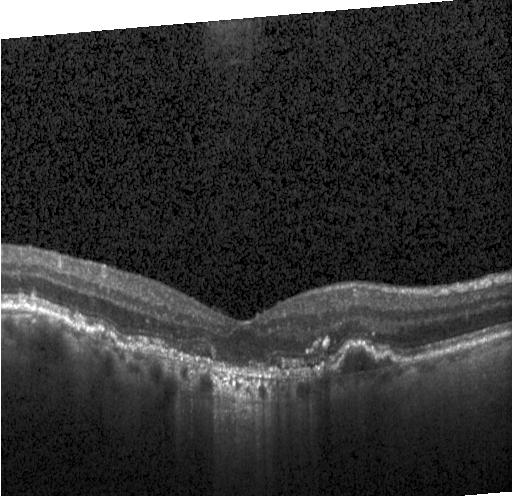 OCT scan showing choroidal neovascularization.